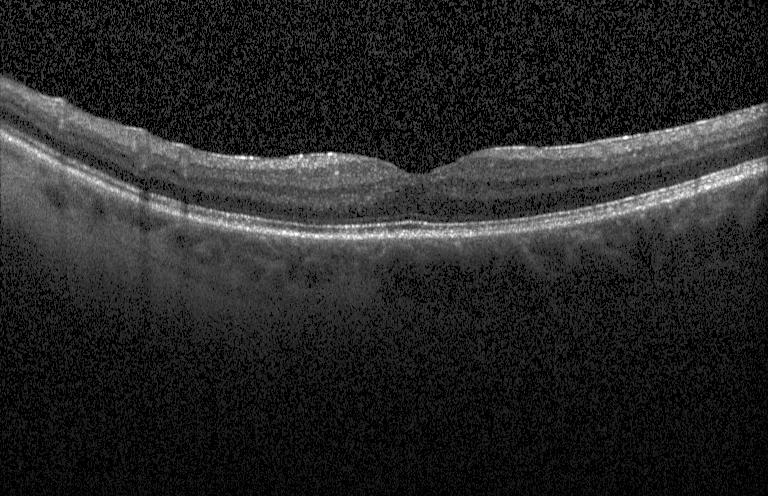

OCT B-scan showing no choroidal neovascularization, no diabetic macular edema, and no drusen.